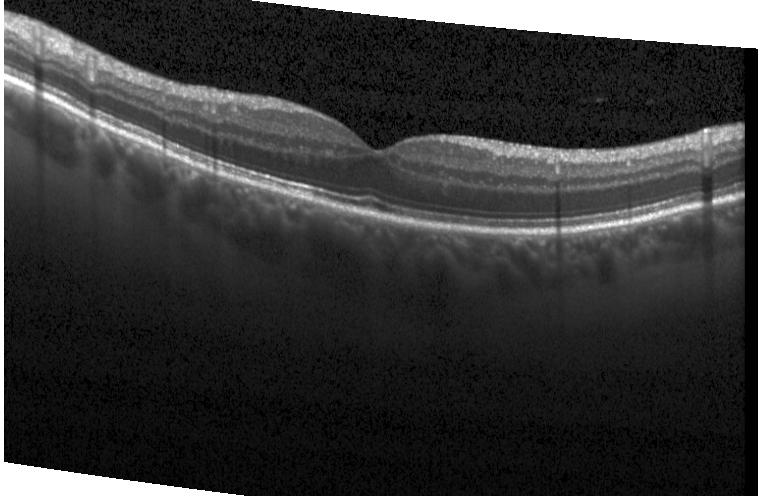

Acquired on a Heidelberg Spectralis, retinal OCT B-scan, through the macula, spectral-domain optical coherence tomography. The scan shows no choroidal neovascularization, no diabetic macular edema, and no drusen.